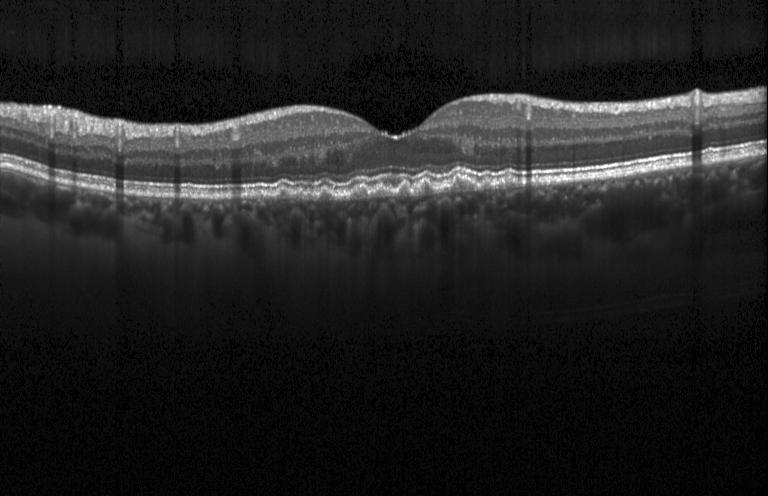 Macular OCT: multiple drusen.